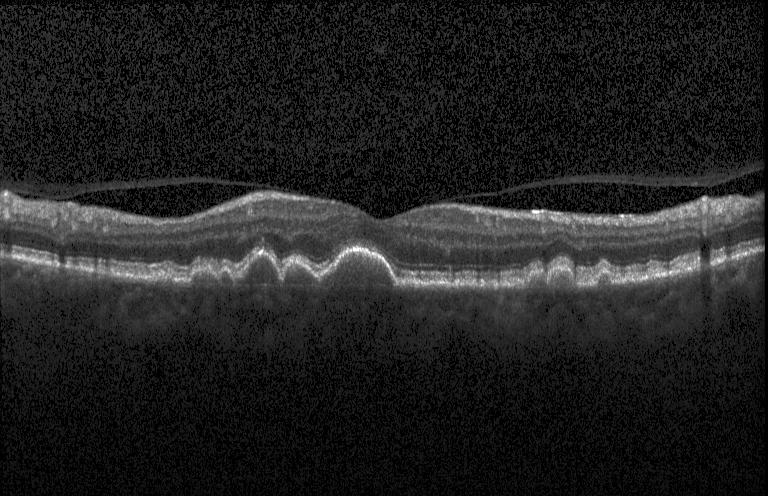

Heidelberg Spectralis · OCT B-scan · spectral-domain OCT.
OCT finding: drusen.